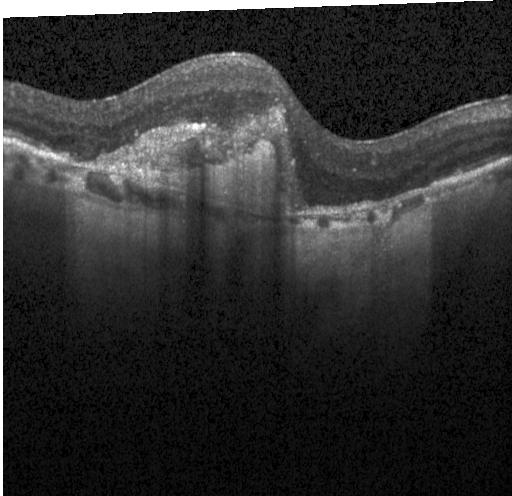
Spectral-domain optical coherence tomography · optical coherence tomography B-scan · Heidelberg Spectralis OCT system
This B-scan demonstrates choroidal neovascularization.